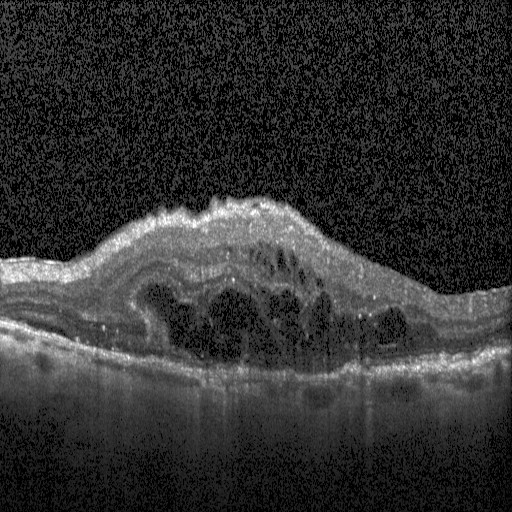

Optical coherence tomography B-scan · instrument: Heidelberg Spectralis · spectral-domain OCT. Diagnosis: diabetic macular edema.